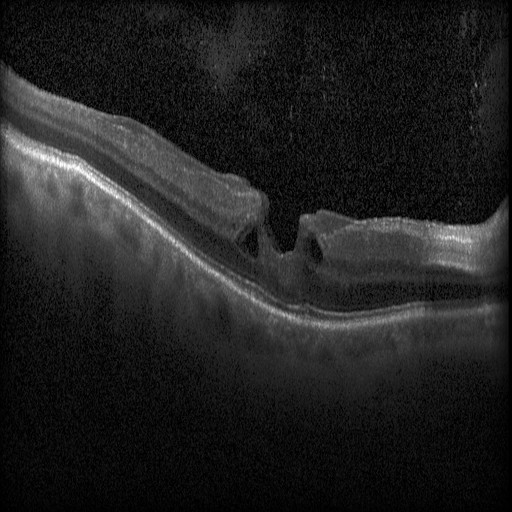

Optical coherence tomography B-scan
This B-scan demonstrates DME.